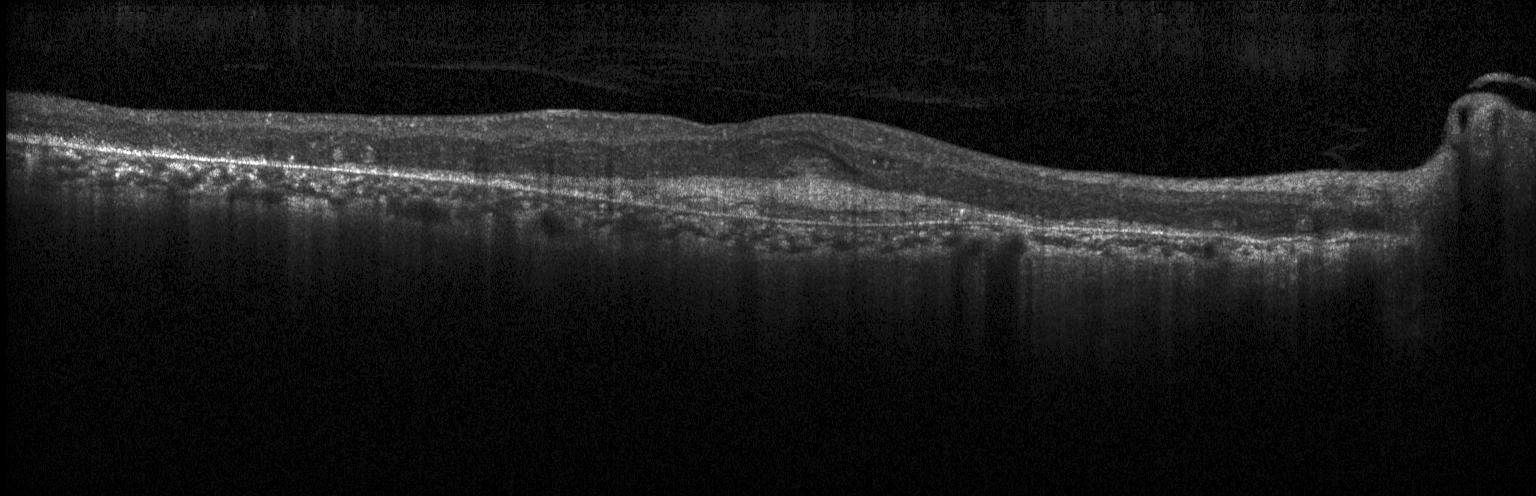
Diagnosis: a choroidal neovascular membrane.